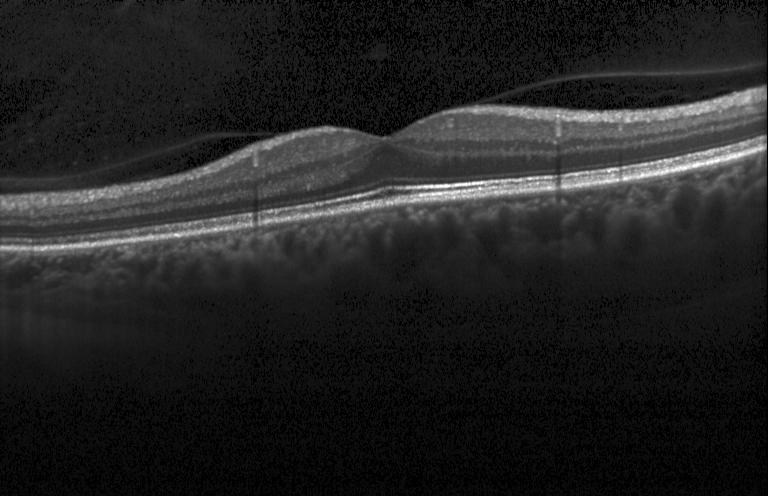 Finding: no evidence of choroidal neovascularization, diabetic macular edema, or drusen.